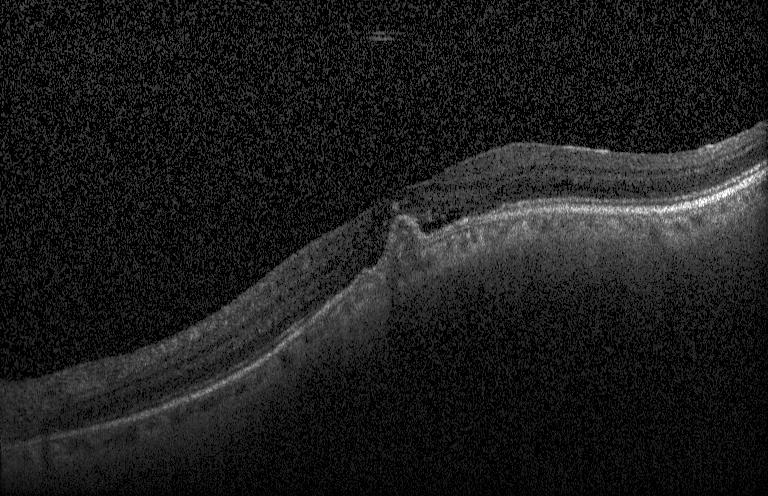 Impression: CNV.